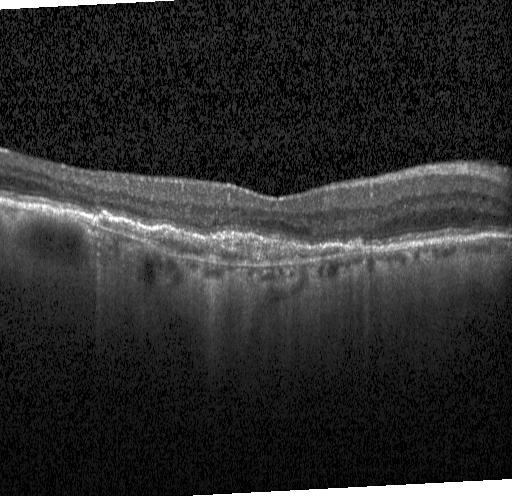 OCT B-scan showing CNV.